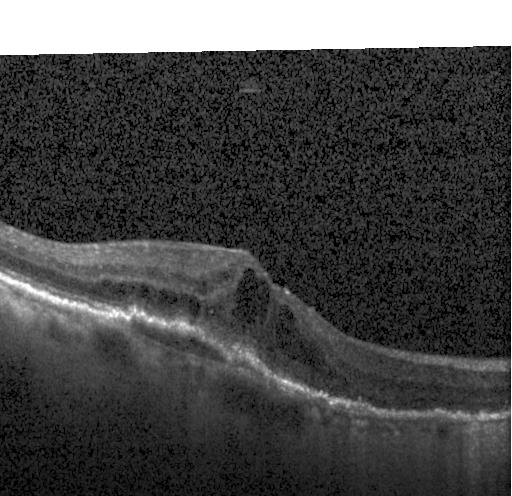 Impression: choroidal neovascularization.